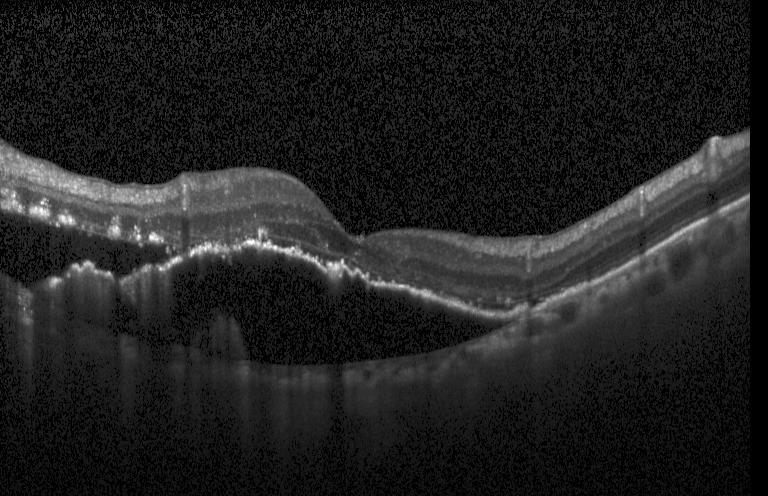 Horizontal scan through the fovea · instrument: Heidelberg Spectralis · OCT line scan
Impression: a choroidal neovascular membrane.